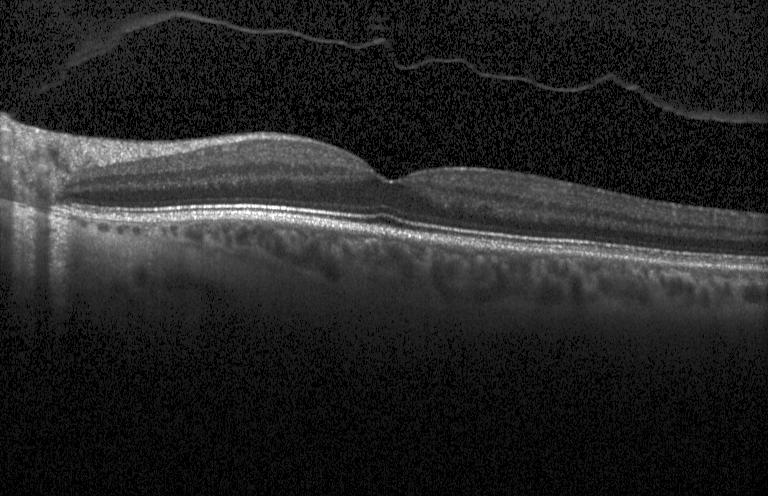
OCT B-scan showing no choroidal neovascularization, no diabetic macular edema, and no drusen.